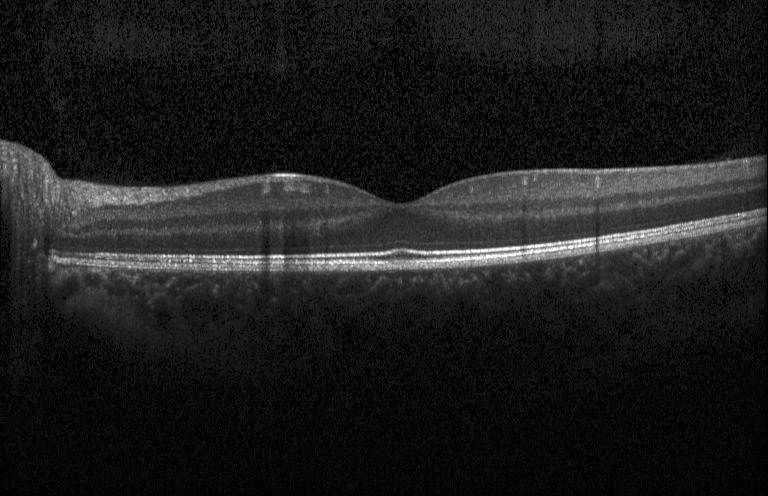 SD-OCT; OCT B-scan
The scan shows no CNV, DME, or drusen.